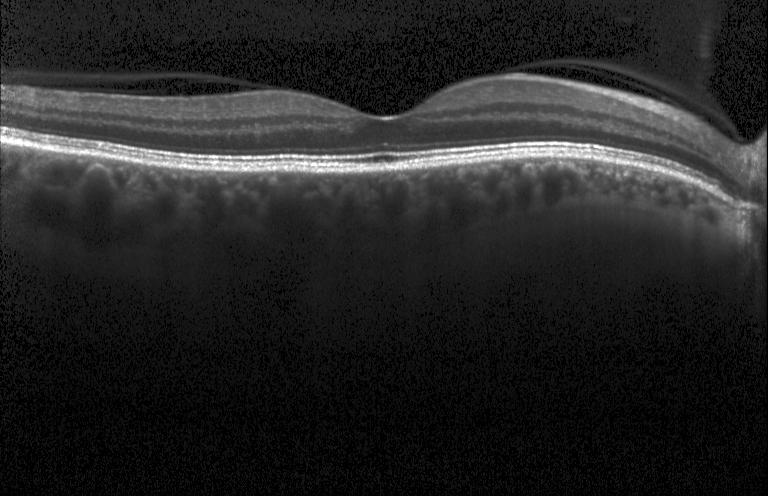 Through the macula. Retinal OCT cross-section. Spectral-domain optical coherence tomography. Impression: no choroidal neovascularization, diabetic macular edema, or drusen.